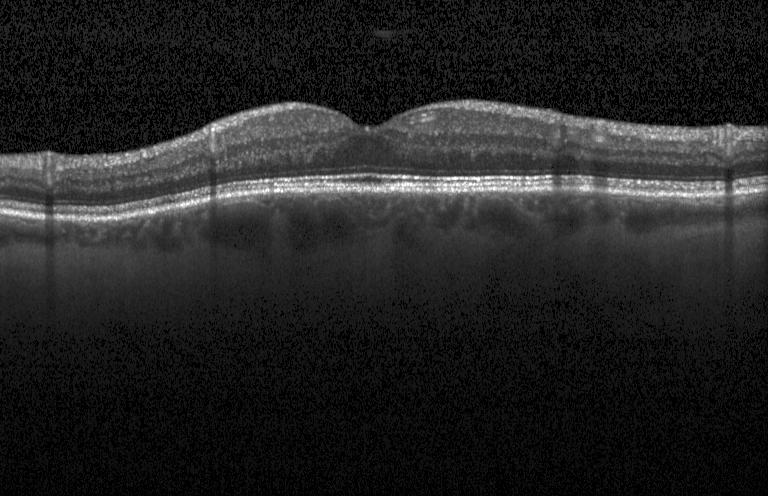 Fovea-centered. OCT B-scan
Macular OCT: no choroidal neovascularization, diabetic macular edema, or drusen.